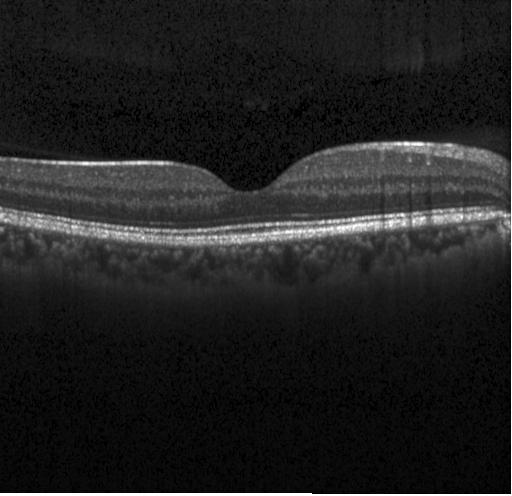
OCT scan showing neither choroidal neovascularization, diabetic macular edema, nor drusen.